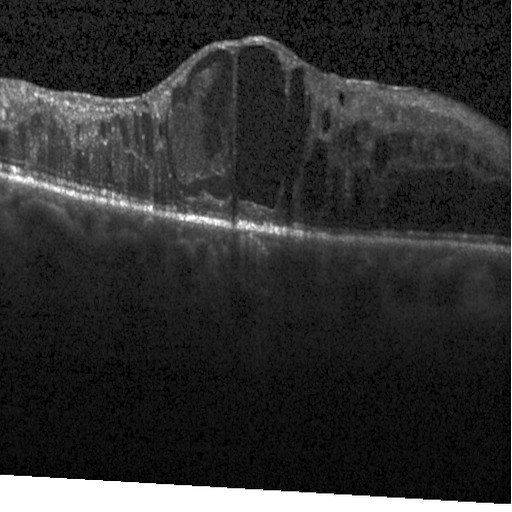
OCT B-scan showing diabetic macular edema.